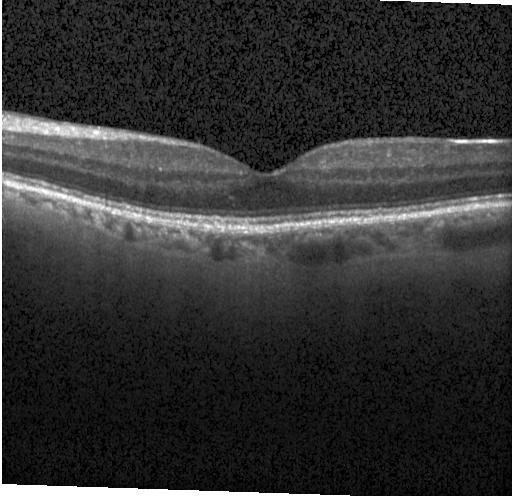 OCT B-scan
Impression: neither choroidal neovascularization, diabetic macular edema, nor drusen.